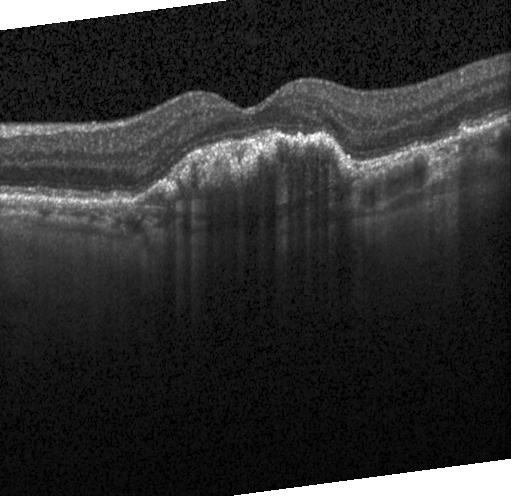

OCT scan showing a choroidal neovascular membrane.